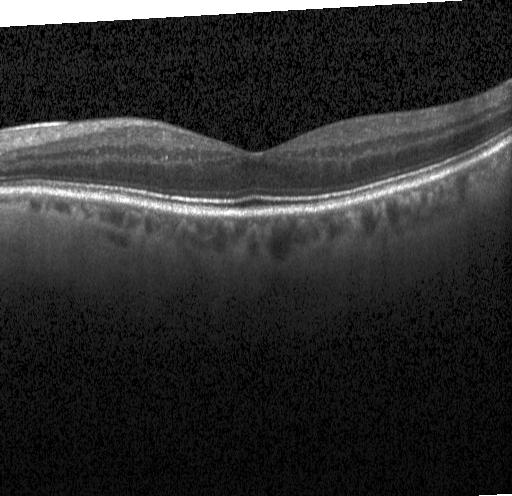
OCT line scan; macular scan
No evidence of choroidal neovascularization, diabetic macular edema, or drusen.